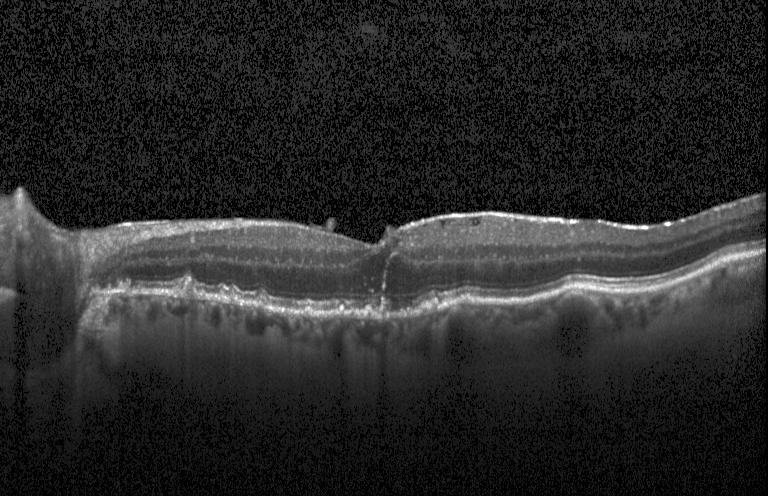 OCT B-scan showing drusen.